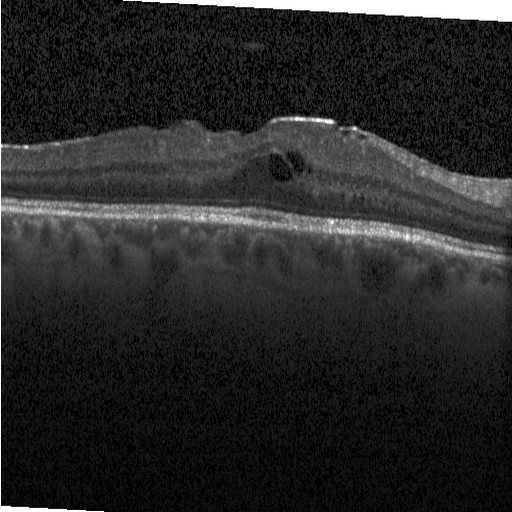 Retinal OCT cross-section. Macular OCT: diabetic macular edema.